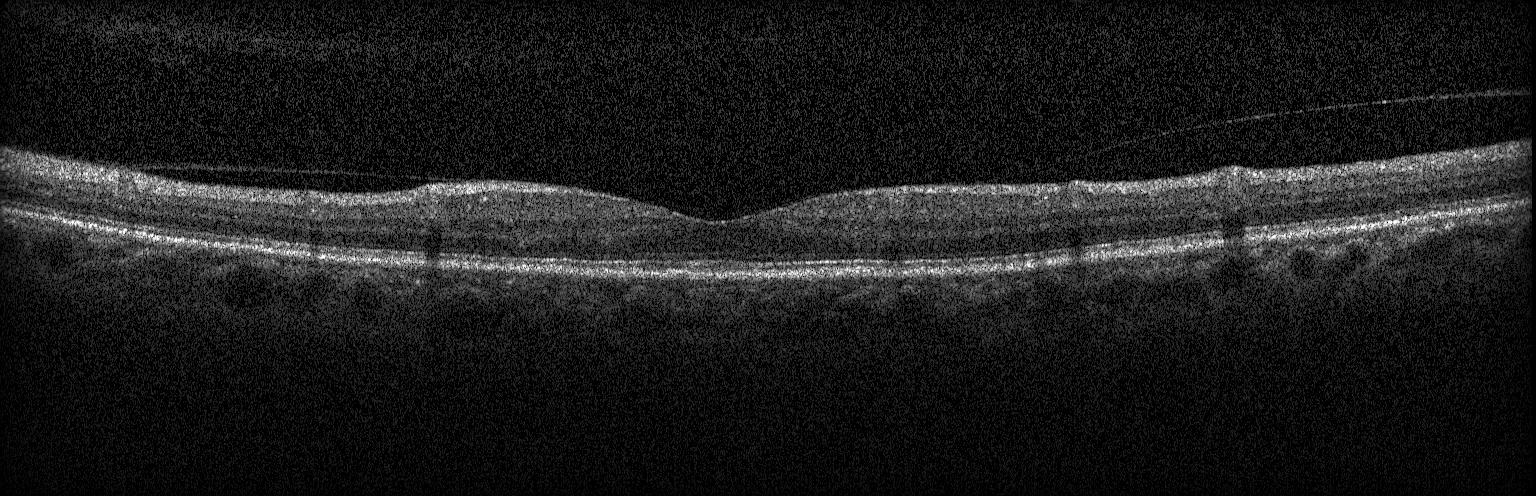

Instrument: Heidelberg Spectralis · macular scan · SD-OCT · OCT B-scan. Finding: no evidence of CNV, DME, or drusen.